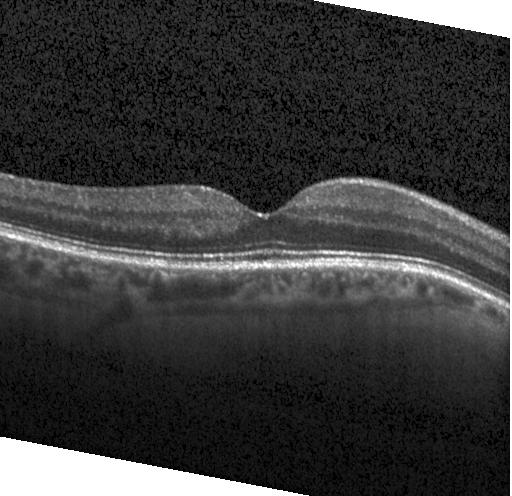
Finding: no evidence of choroidal neovascularization, diabetic macular edema, or drusen.